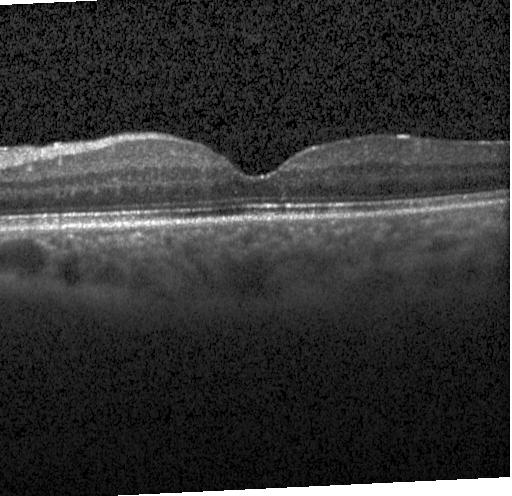

Horizontal scan through the fovea; spectral-domain optical coherence tomography; retinal OCT B-scan; Heidelberg Spectralis OCT system. Diagnosis: no evidence of CNV, DME, or drusen.